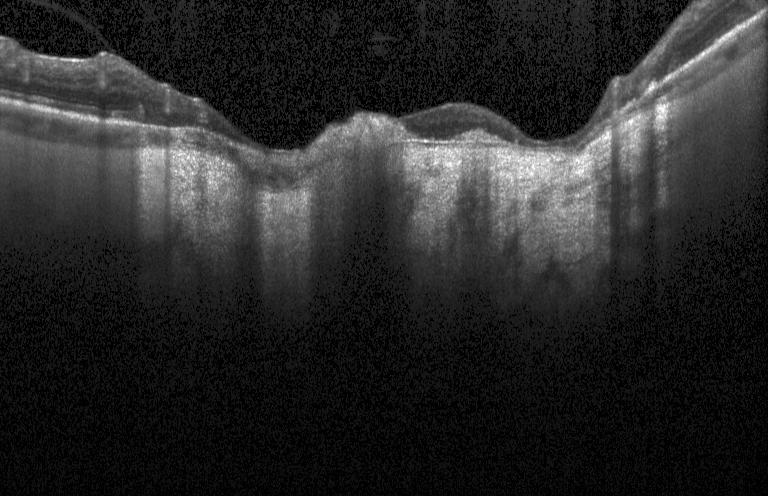 Finding: choroidal neovascularization.